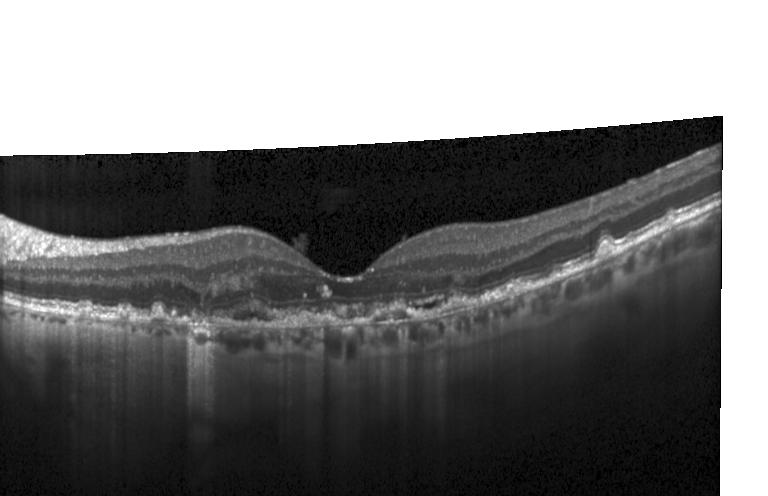
OCT finding: CNV.